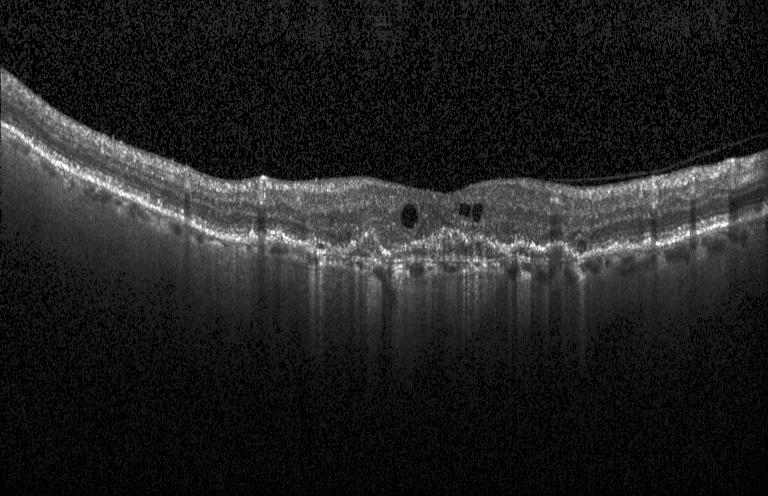

Spectral-domain OCT B-scan: a choroidal neovascular membrane.